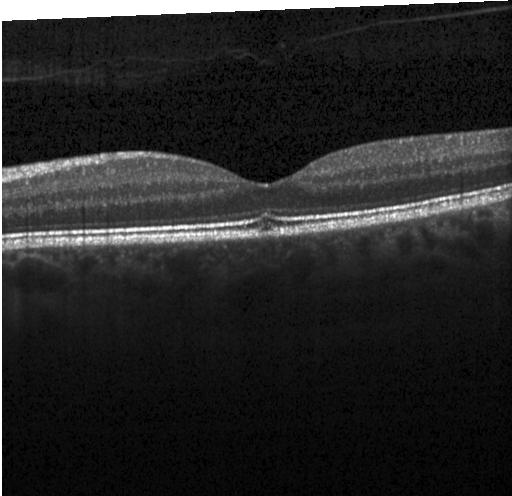

No choroidal neovascularization, no diabetic macular edema, and no drusen.